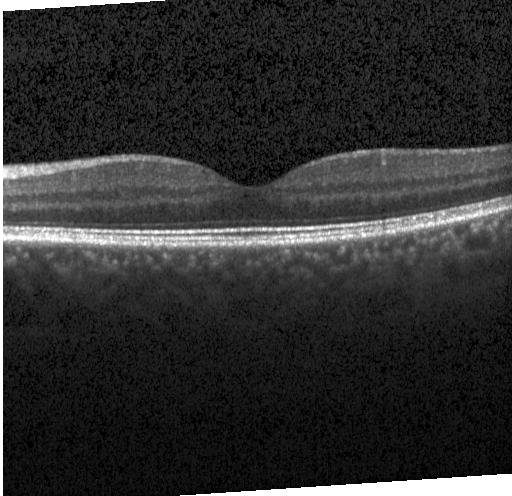

Macular scan · spectral-domain OCT · retinal OCT B-scan
Dx: no choroidal neovascularization, diabetic macular edema, or drusen.